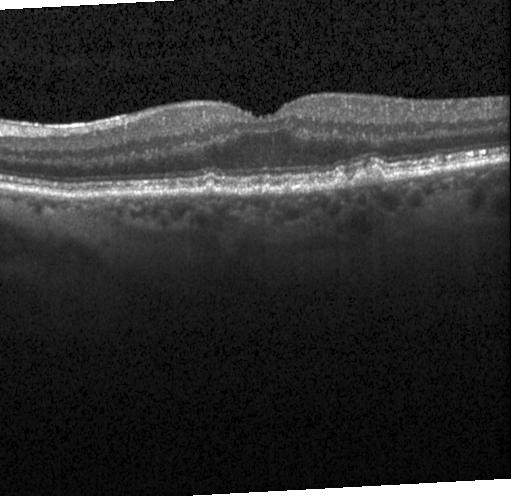
Dx: sub-RPE drusenoid deposits.